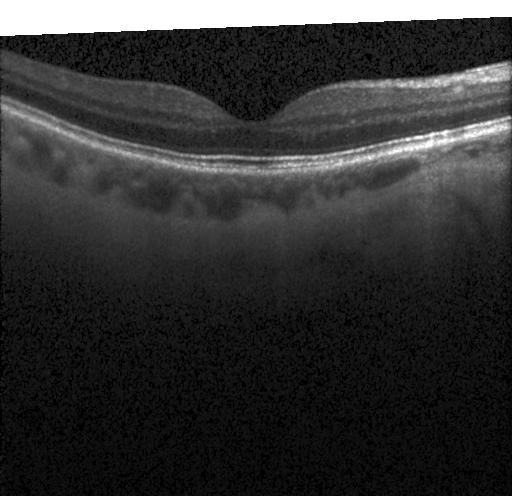

Retinal OCT B-scan
Diagnosis: neither CNV, DME, nor drusen.